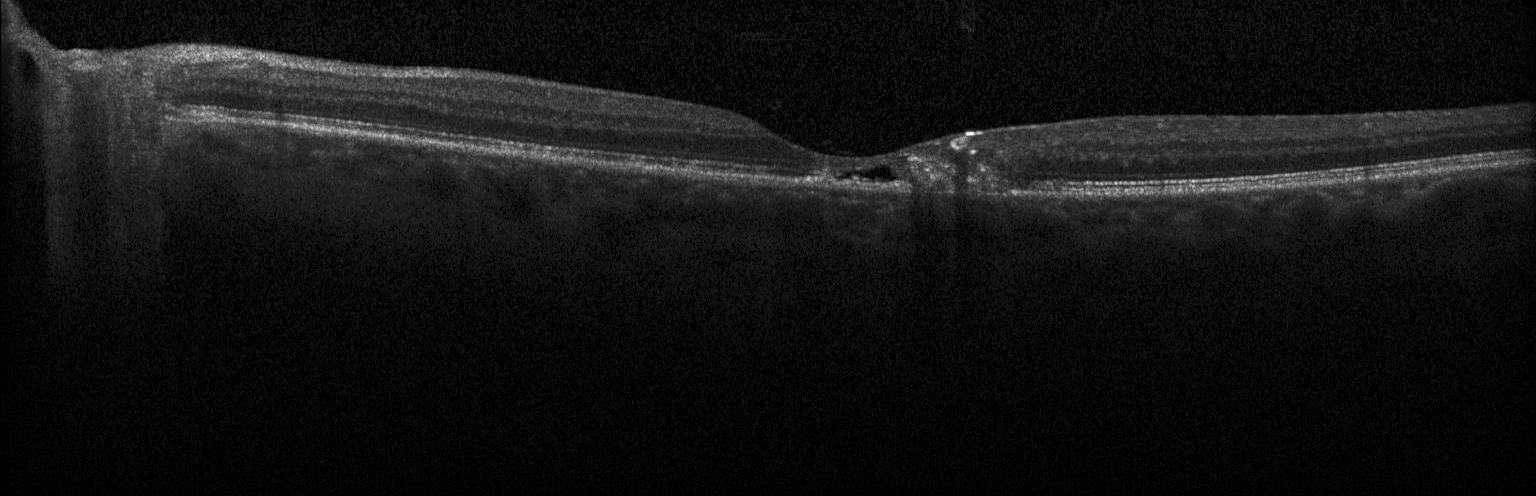 Impression: CNV.